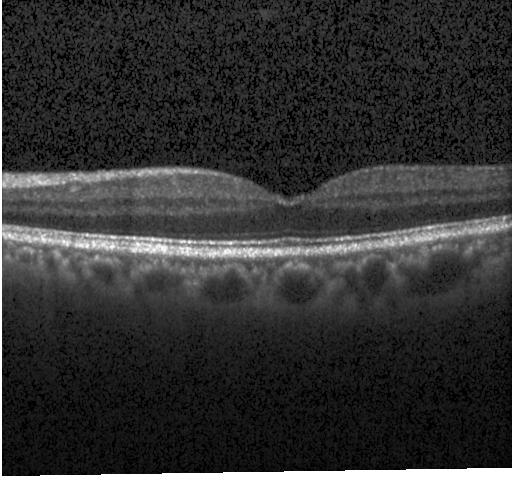 OCT B-scan. Finding: neither CNV, DME, nor drusen.